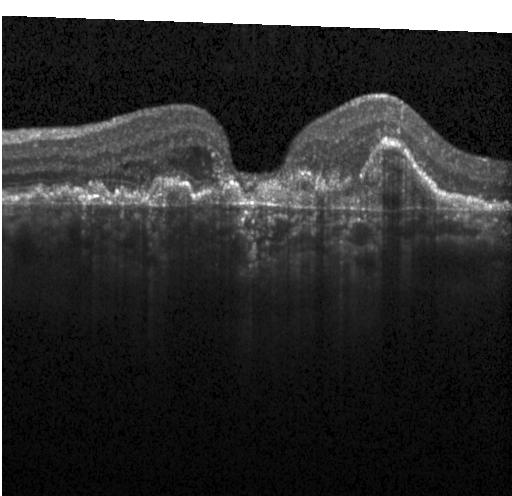

OCT line scan. Heidelberg Spectralis. Fovea-centered
Impression: choroidal neovascularization.